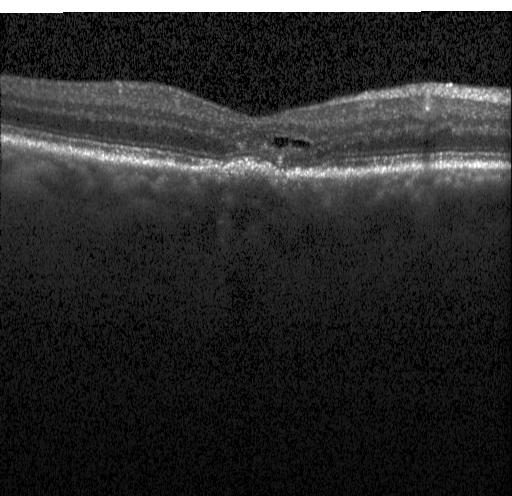
CNV.